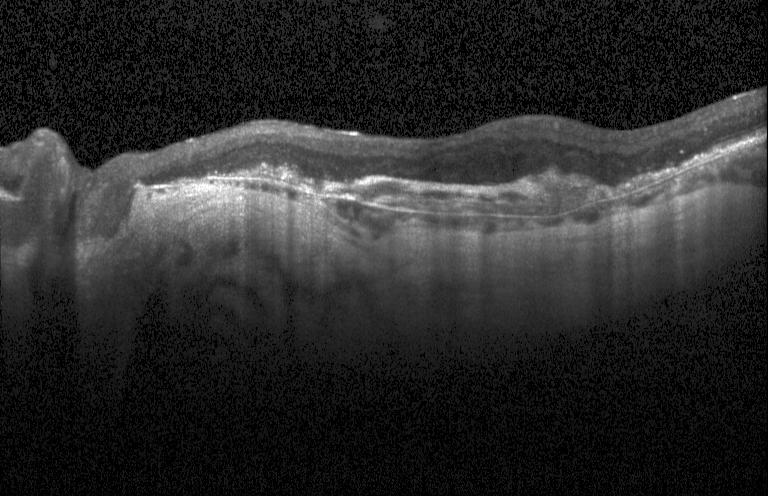
The scan shows a choroidal neovascular membrane.